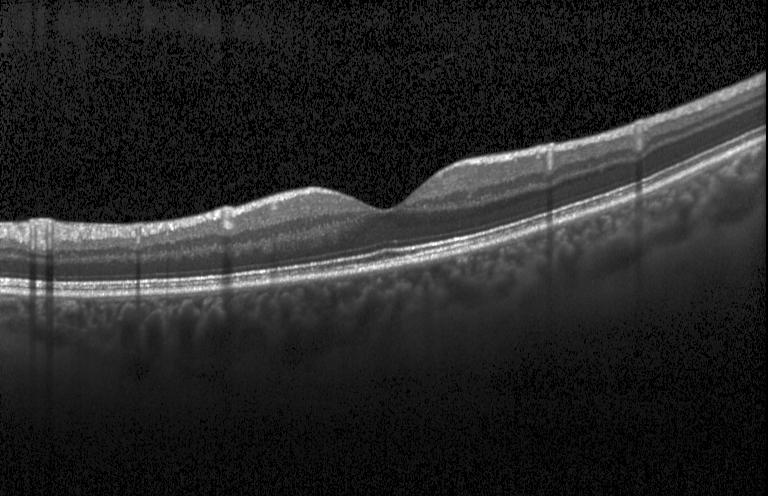 Heidelberg Spectralis OCT system · centered on the fovea · OCT line scan · spectral-domain OCT — Assessment: no CNV, no DME, and no drusen.